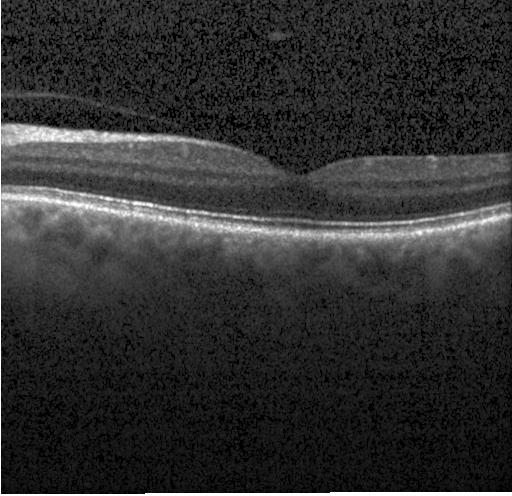 Spectral-domain optical coherence tomography, retinal OCT cross-section, macular scan, instrument: Heidelberg Spectralis — Impression: neither choroidal neovascularization, diabetic macular edema, nor drusen.